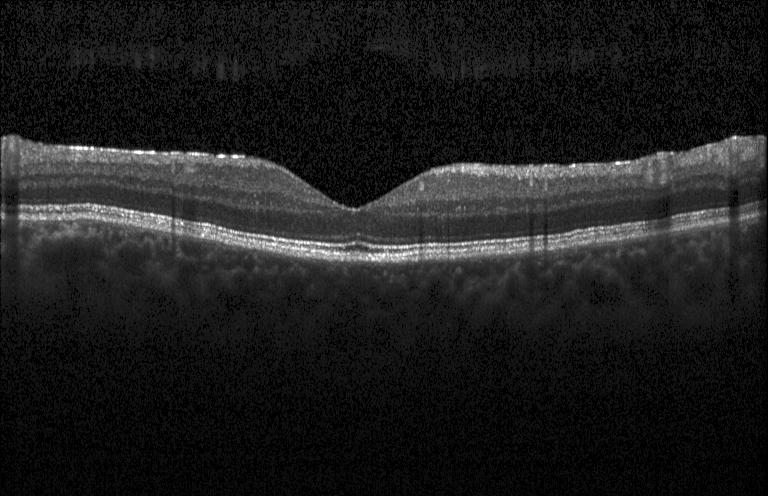

Acquired on a Heidelberg Spectralis; OCT B-scan. Impression: no CNV, no DME, and no drusen.